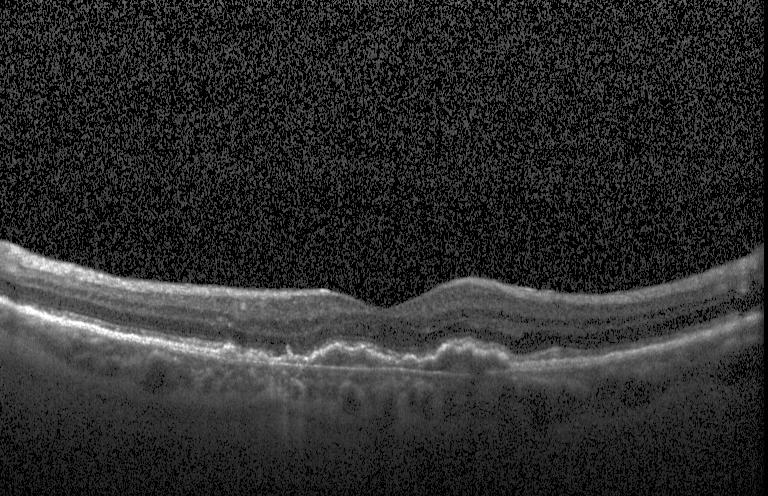 Heidelberg Spectralis OCT system · fovea-centered · OCT line scan
Finding: choroidal neovascularization.